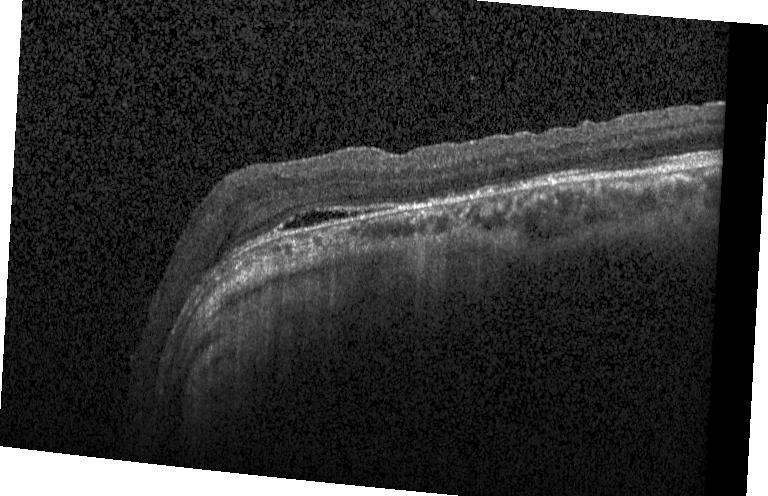

Through the macula · SD-OCT · optical coherence tomography B-scan. Impression: CNV.